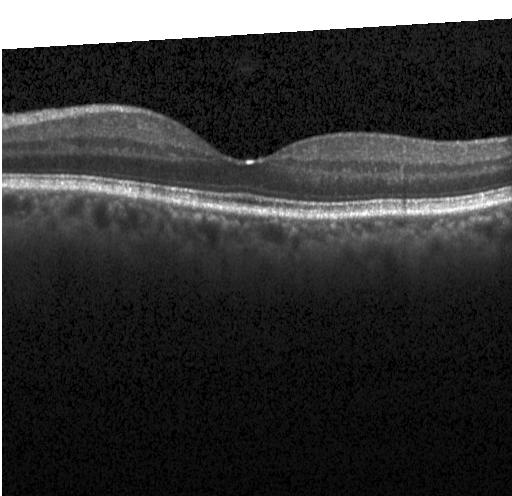

Retinal OCT B-scan; through the macula; spectral-domain OCT — Assessment: no choroidal neovascularization, diabetic macular edema, or drusen.